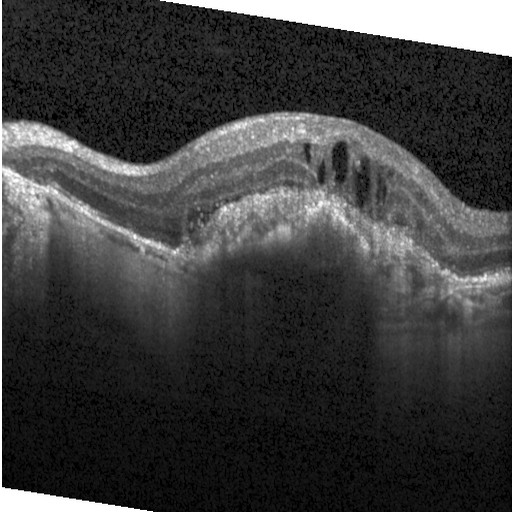 Dx: diabetic macular edema (DME).